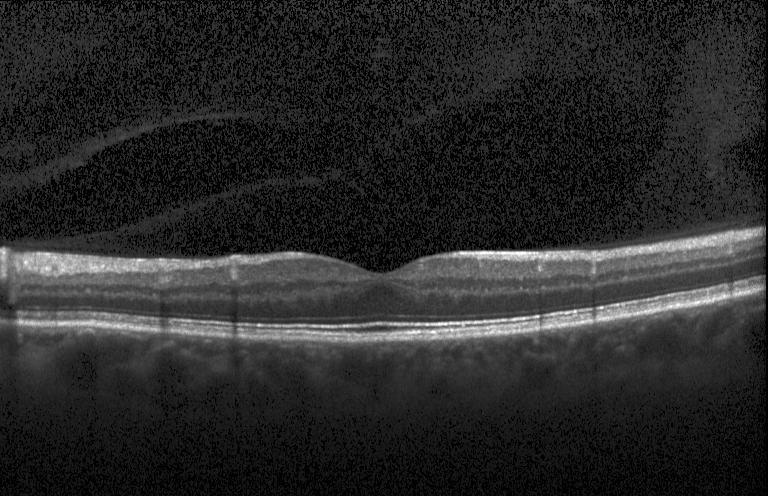 Finding: no evidence of choroidal neovascularization, diabetic macular edema, or drusen.